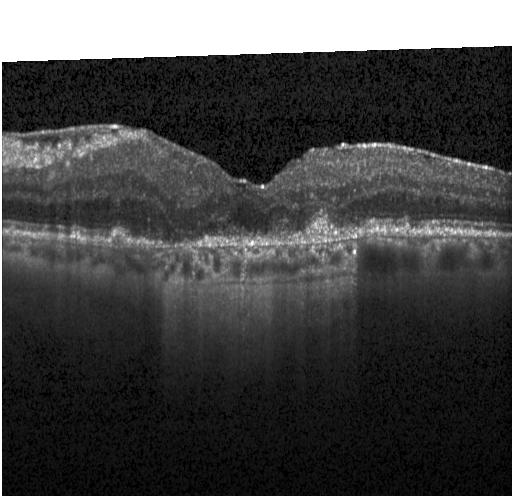 SD-OCT · retinal OCT B-scan. Diagnosis: a choroidal neovascular membrane.